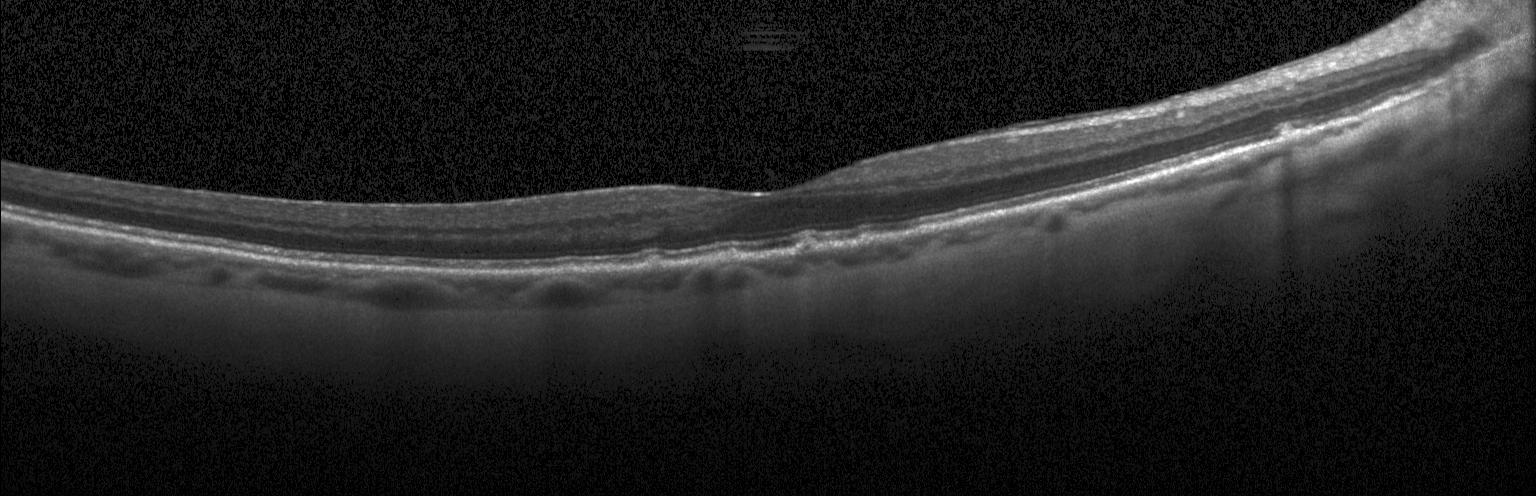 OCT line scan, SD-OCT, fovea-centered
Impression: multiple drusen.